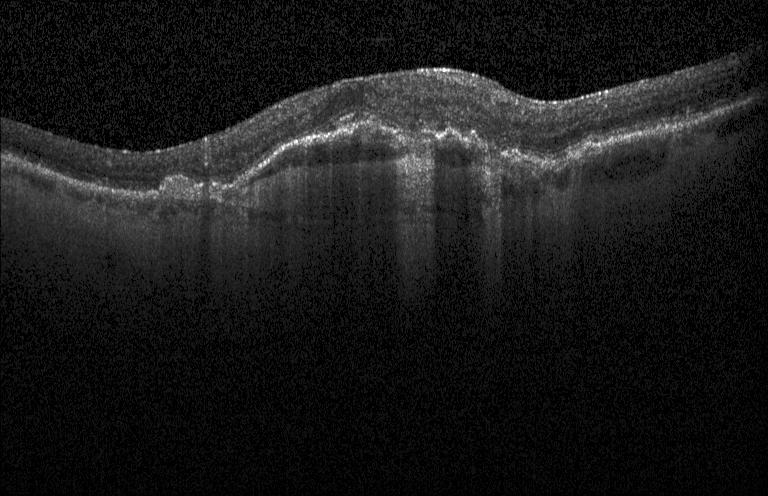
Diagnosis: a choroidal neovascular membrane.